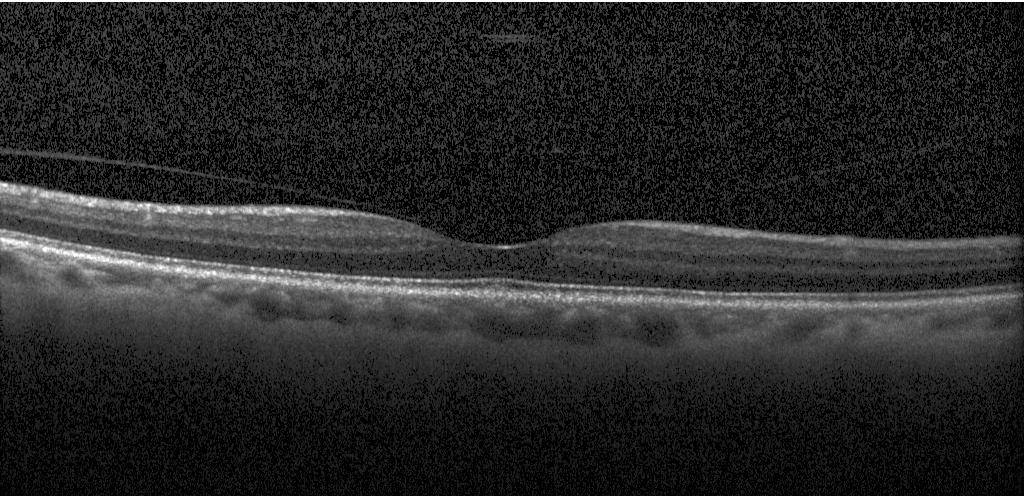

Retinal OCT cross-section — Finding: no evidence of CNV, DME, or drusen.